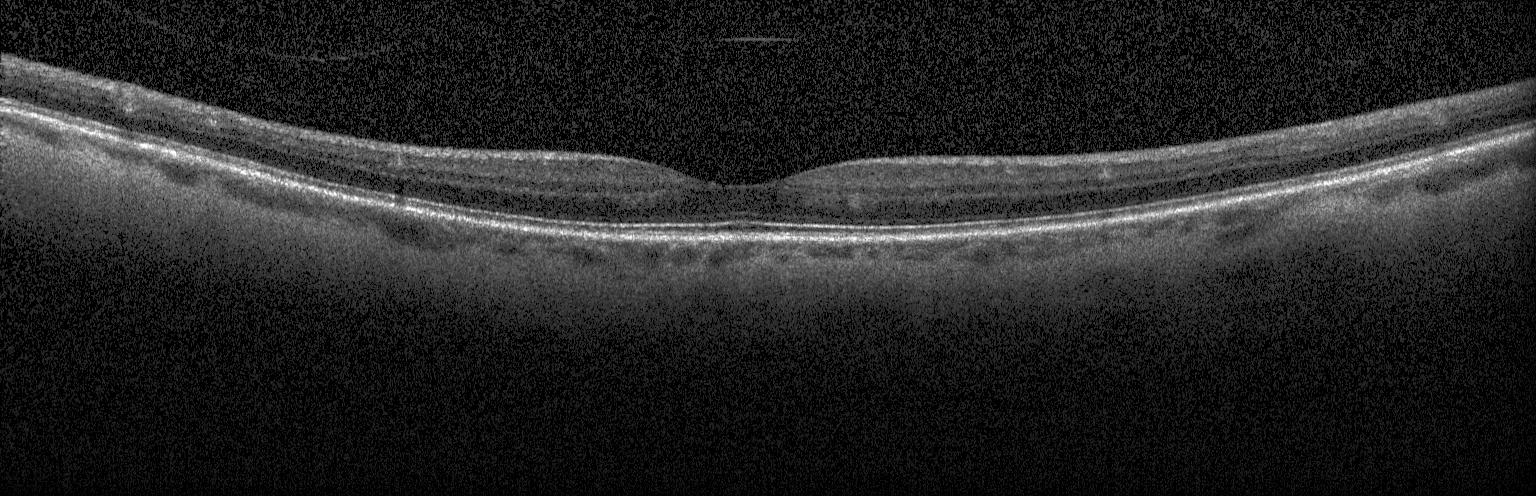
Retinal OCT B-scan · spectral-domain optical coherence tomography — Finding: no choroidal neovascularization, no diabetic macular edema, and no drusen.